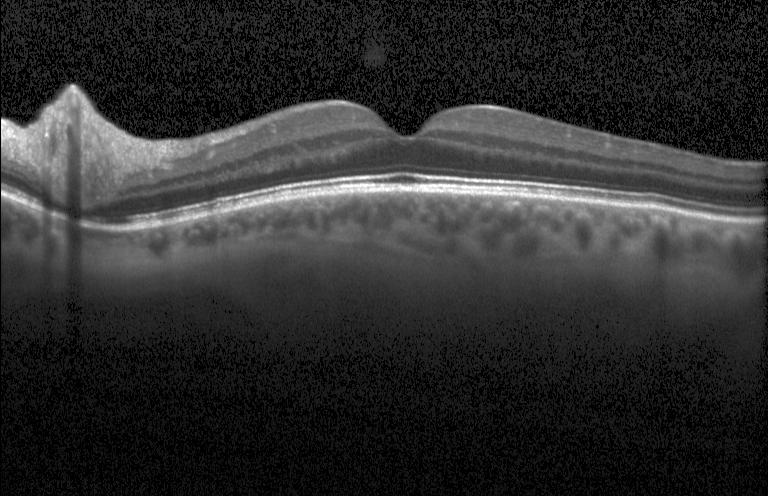 Heidelberg Spectralis, SD-OCT, through the macula, OCT line scan — No evidence of CNV, DME, or drusen.